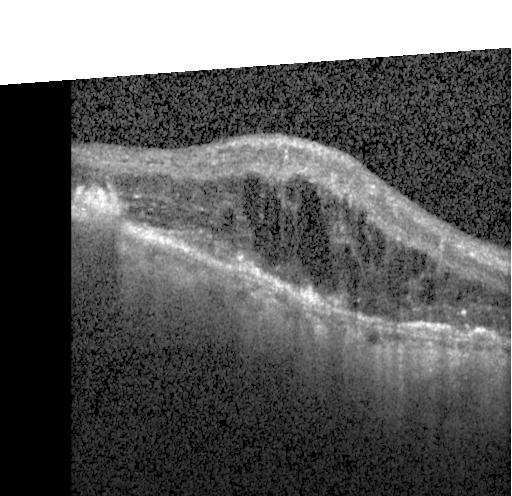 OCT finding: a choroidal neovascular membrane.